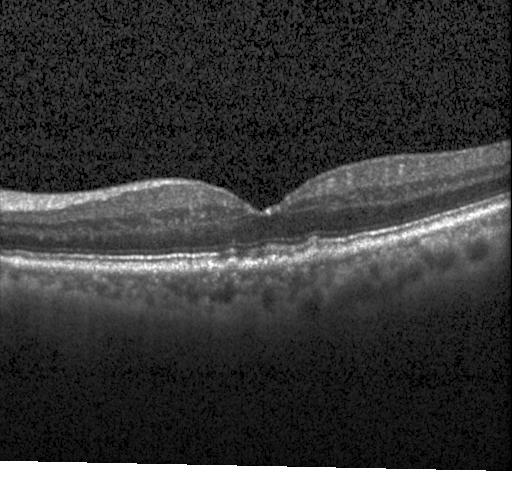

Retinal OCT B-scan.
Sub-RPE drusenoid deposits.